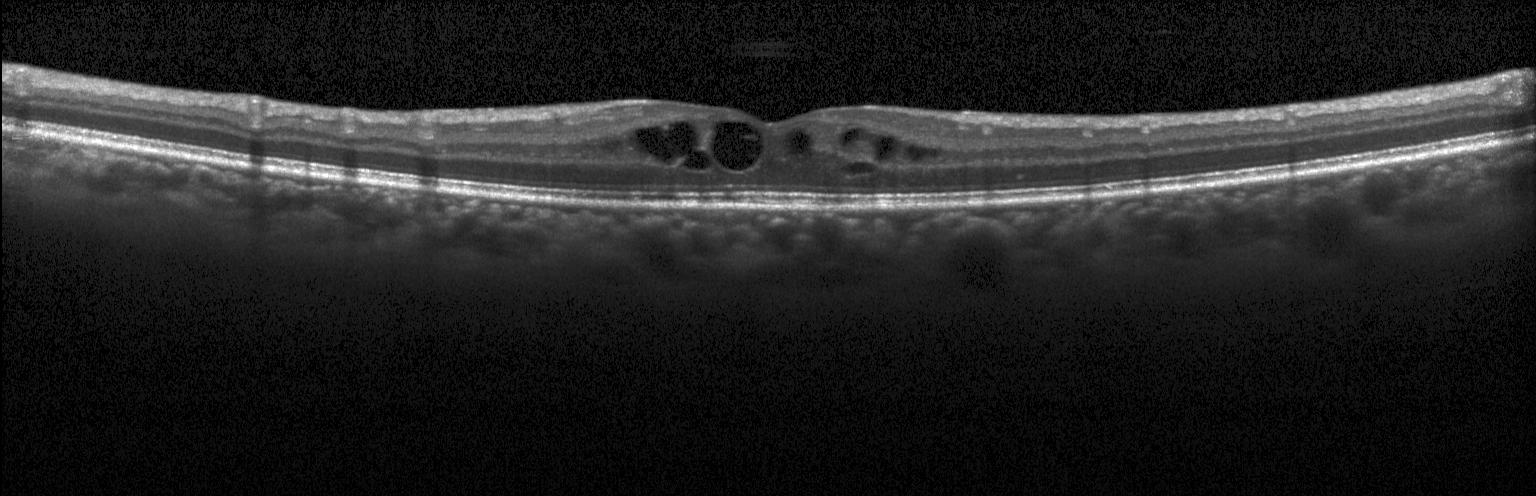
The scan shows diabetic macular edema (DME).